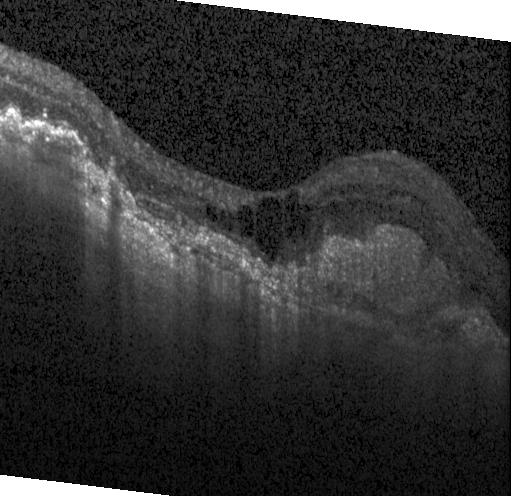

Diagnosis: a choroidal neovascular membrane.